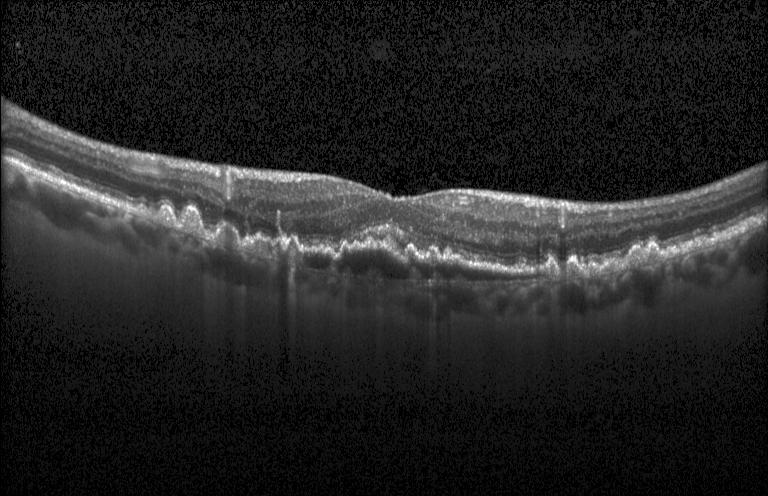 OCT line scan, macular scan, instrument: Heidelberg Spectralis. Finding: a choroidal neovascular membrane.